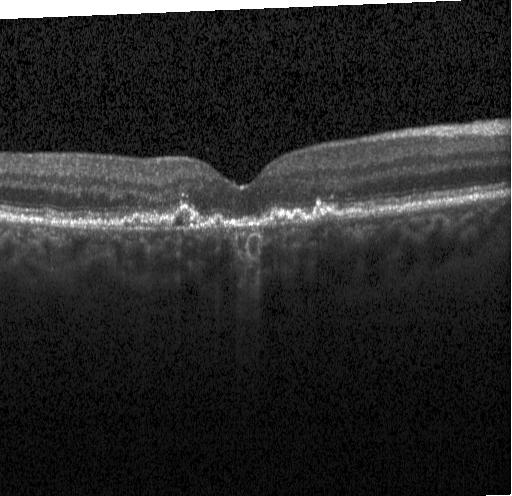 OCT finding: CNV.